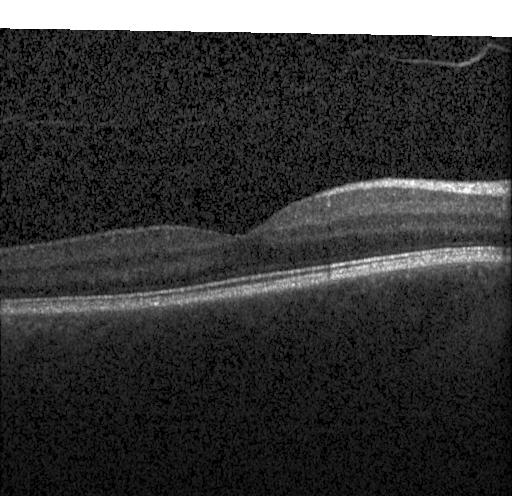
Retinal OCT cross-section, SD-OCT. This B-scan demonstrates no CNV, DME, or drusen.